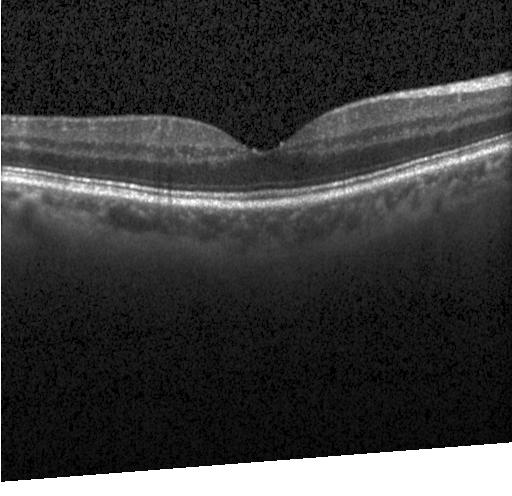

Impression: no CNV, DME, or drusen.